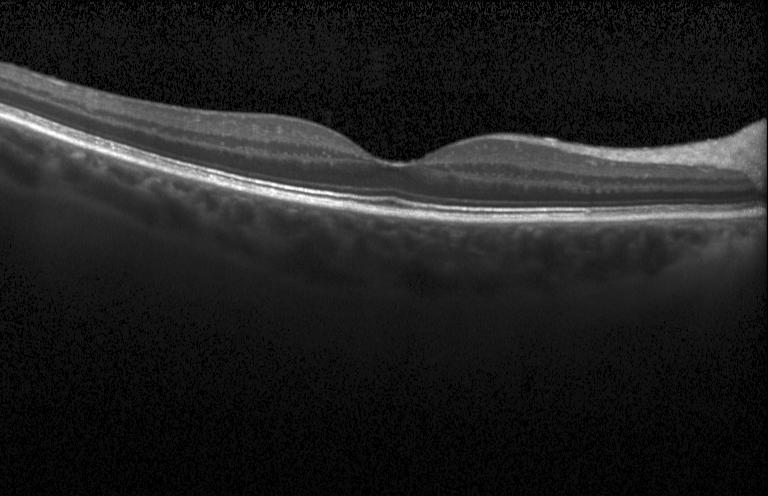 OCT B-scan.
Macular OCT: no choroidal neovascularization, no diabetic macular edema, and no drusen.